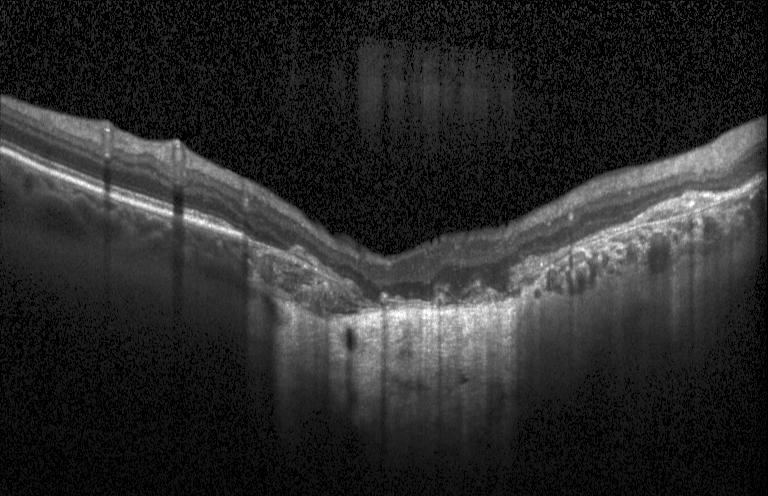

Macular OCT demonstrating a choroidal neovascular membrane.